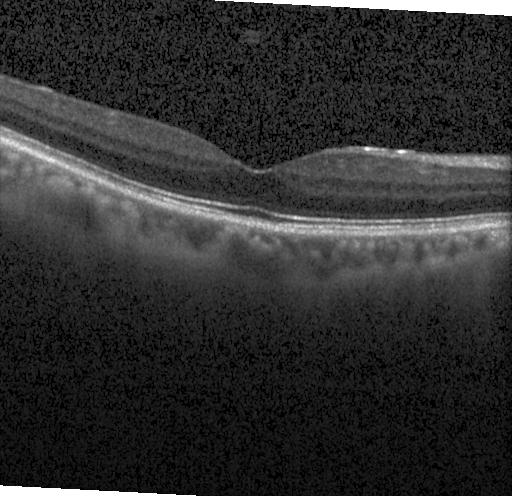 Retinal OCT cross-section.
Diagnosis: no choroidal neovascularization, diabetic macular edema, or drusen.